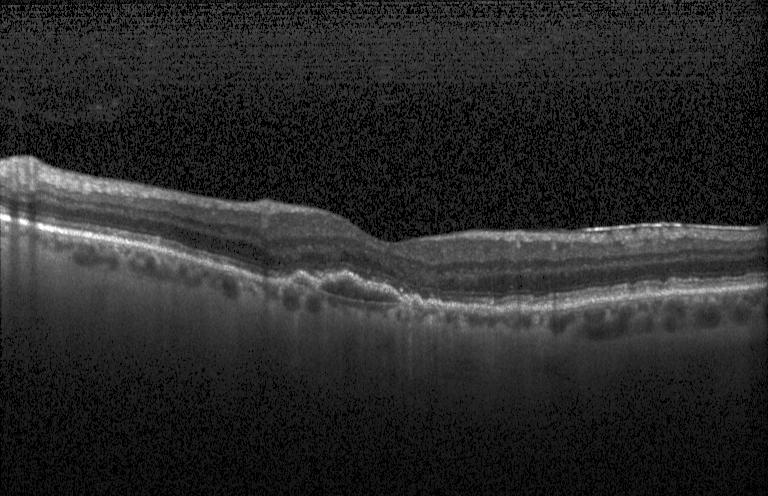
Retinal OCT cross-section · fovea-centered. OCT finding: choroidal neovascularization (CNV).